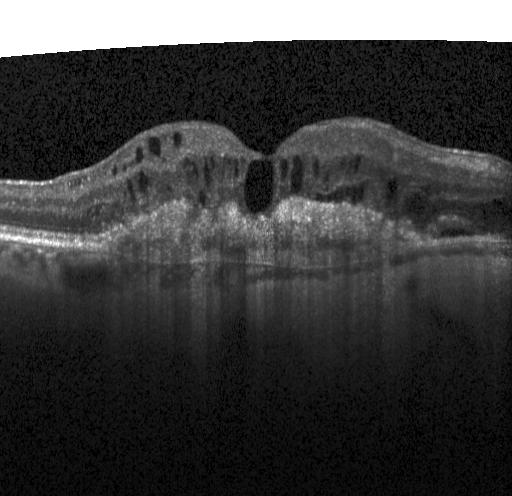

The scan shows CNV.